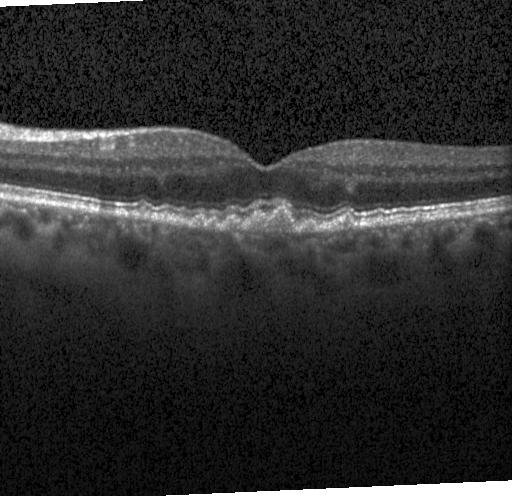 Drusen.